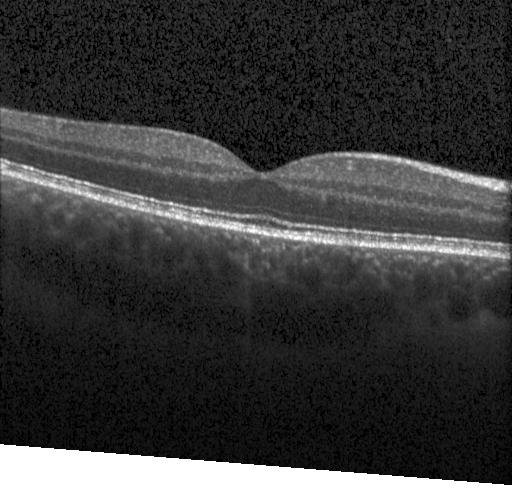 Instrument: Heidelberg Spectralis. Macular scan. SD-OCT. Optical coherence tomography scan.
No choroidal neovascularization, diabetic macular edema, or drusen.